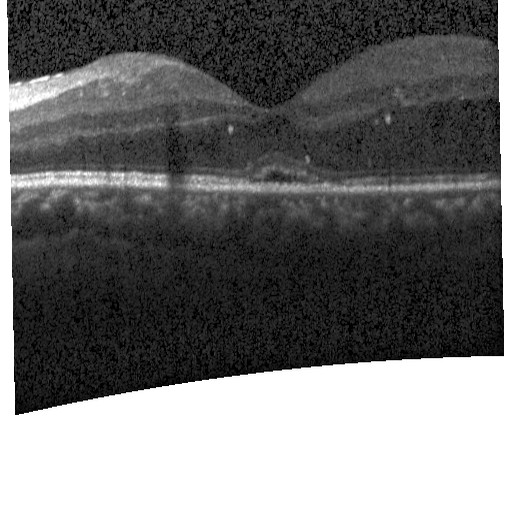 Diagnosis: diabetic macular edema (DME).